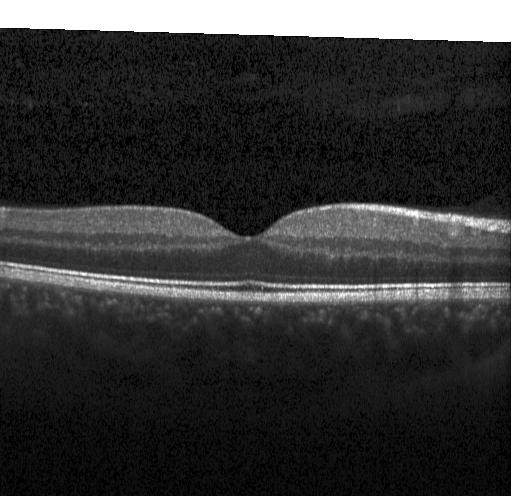
Retinal OCT B-scan.
No choroidal neovascularization, no diabetic macular edema, and no drusen.